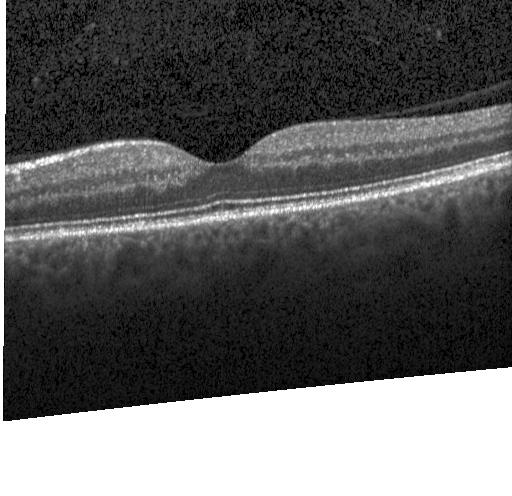

Centered on the fovea · OCT B-scan · spectral-domain optical coherence tomography · Heidelberg Spectralis OCT system
Finding: neither choroidal neovascularization, diabetic macular edema, nor drusen.